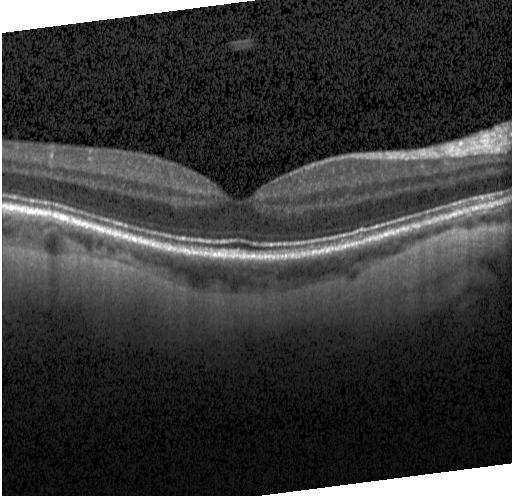

OCT B-scan.
OCT finding: no CNV, DME, or drusen.